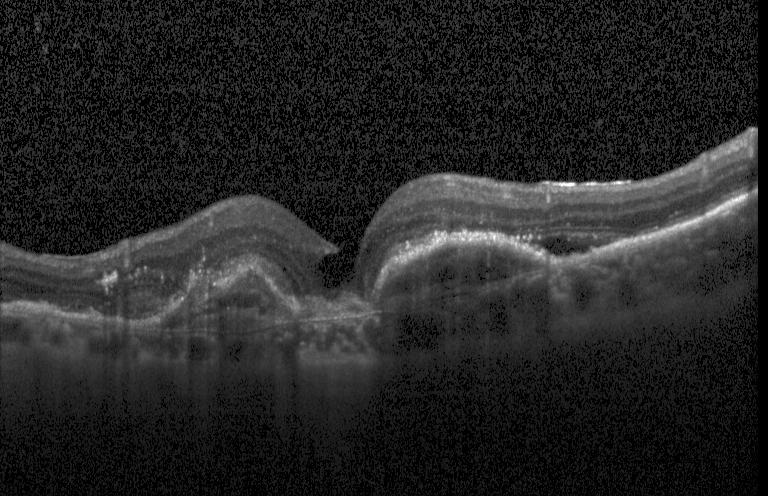
Impression: CNV.